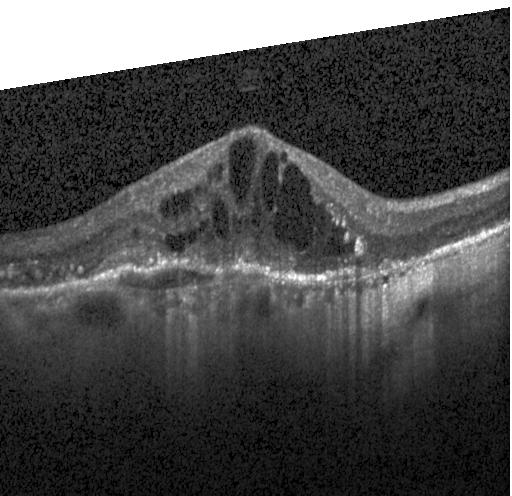 Impression: CNV.